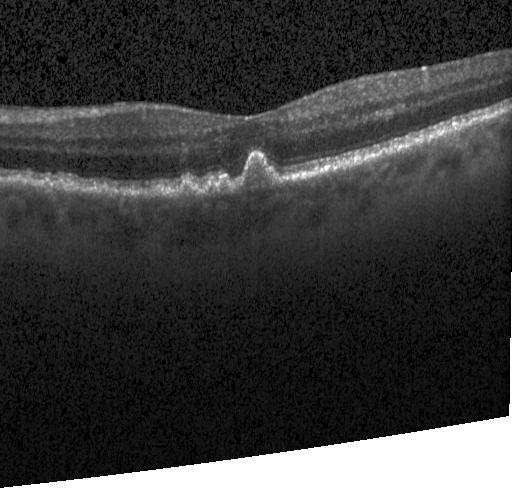

Optical coherence tomography B-scan.
Finding: drusen.